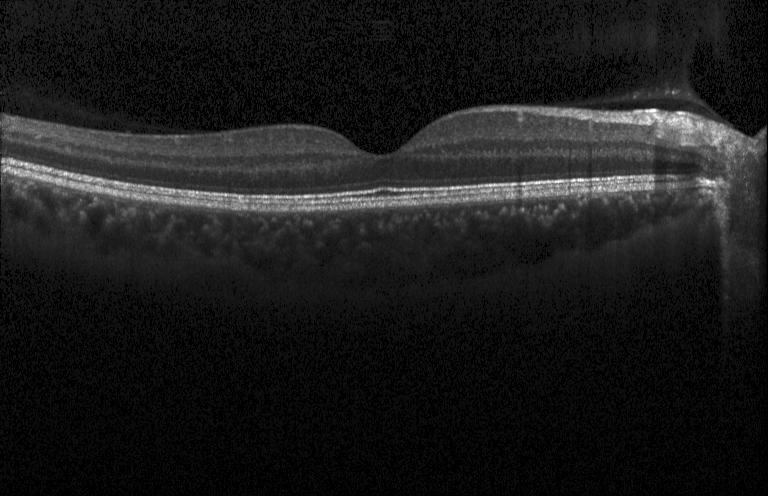 Spectral-domain optical coherence tomography. Heidelberg Spectralis OCT system. OCT line scan — Macular OCT: no choroidal neovascularization, no diabetic macular edema, and no drusen.